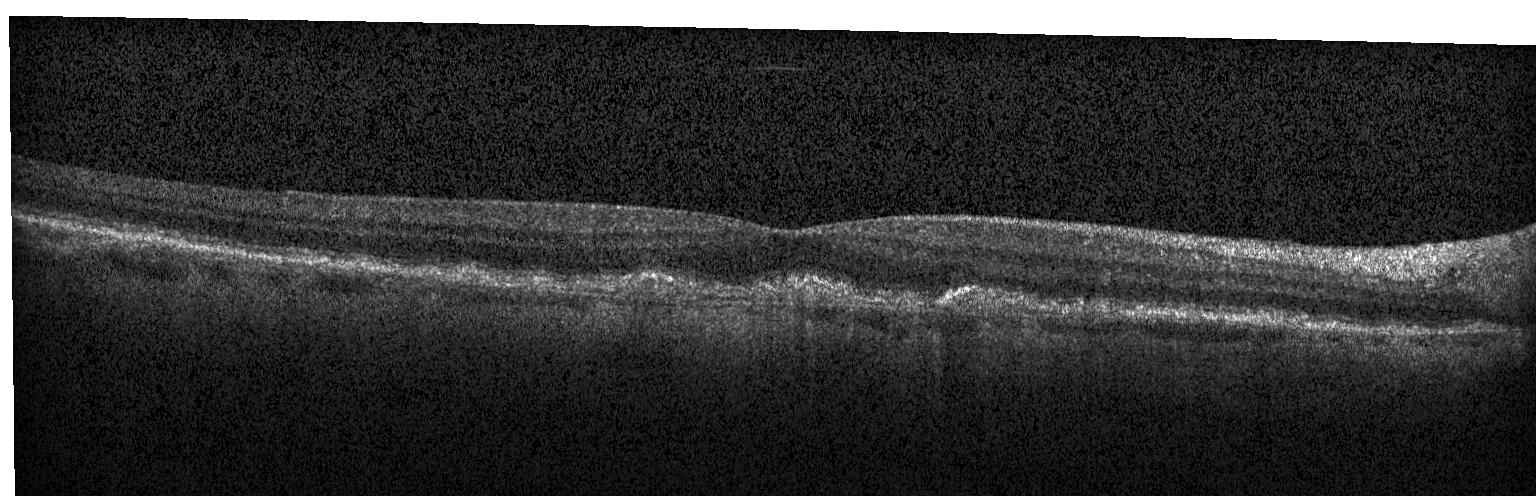

Spectral-domain optical coherence tomography, acquired on a Heidelberg Spectralis, optical coherence tomography scan, through the macula. Diagnosis: a choroidal neovascular membrane.